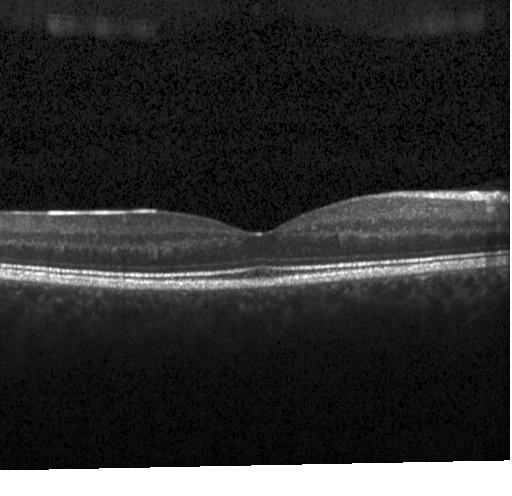

Retinal OCT cross-section showing no choroidal neovascularization, no diabetic macular edema, and no drusen.